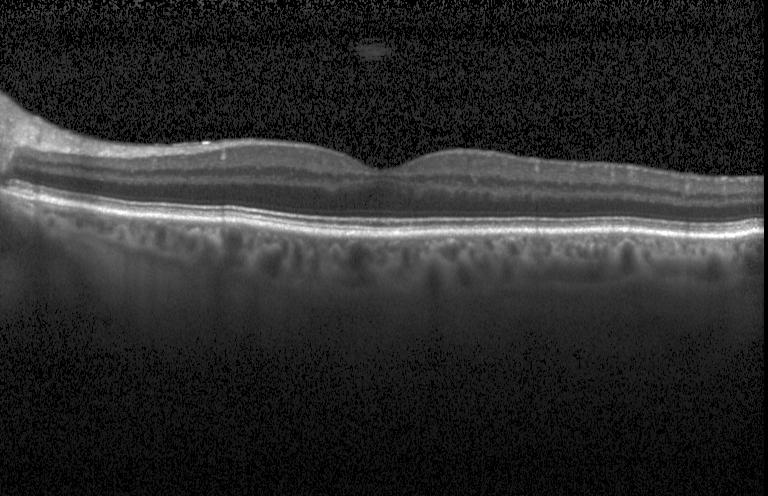

Diagnosis: no evidence of CNV, DME, or drusen.